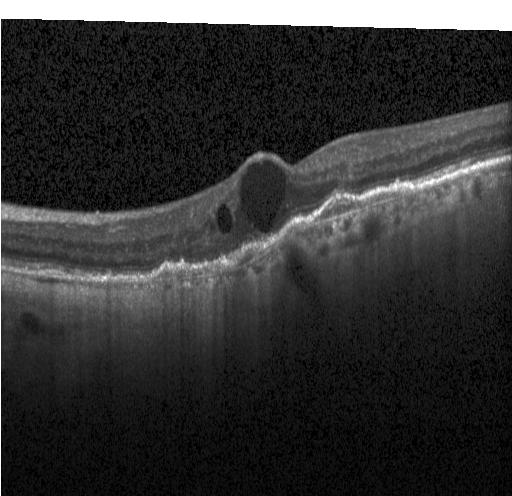
Heidelberg Spectralis OCT system · OCT line scan · spectral-domain OCT
Impression: a choroidal neovascular membrane.